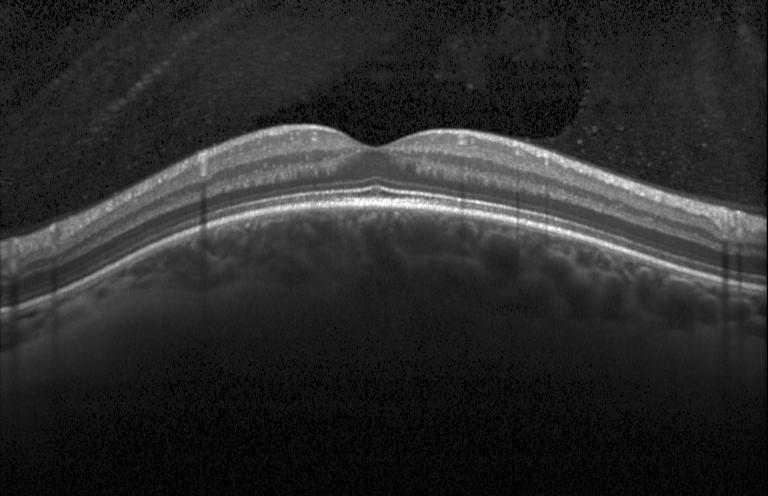

Retinal OCT B-scan, fovea-centered, acquired on a Heidelberg Spectralis.
OCT finding: no choroidal neovascularization, no diabetic macular edema, and no drusen.